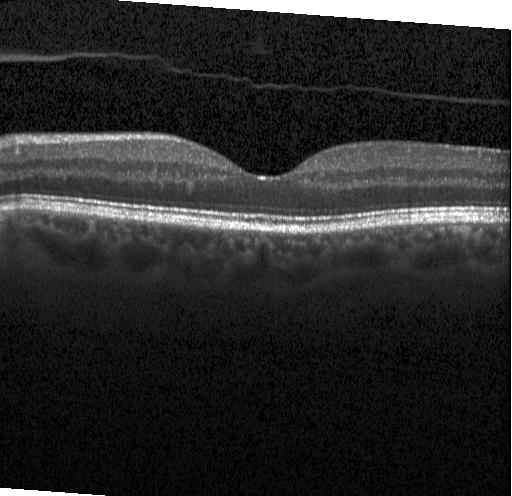
Heidelberg Spectralis OCT system. OCT line scan. The scan shows no evidence of CNV, DME, or drusen.